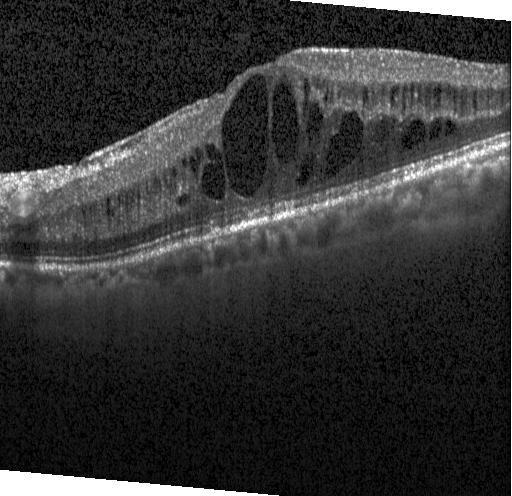
Retinal OCT B-scan.
Impression: DME.